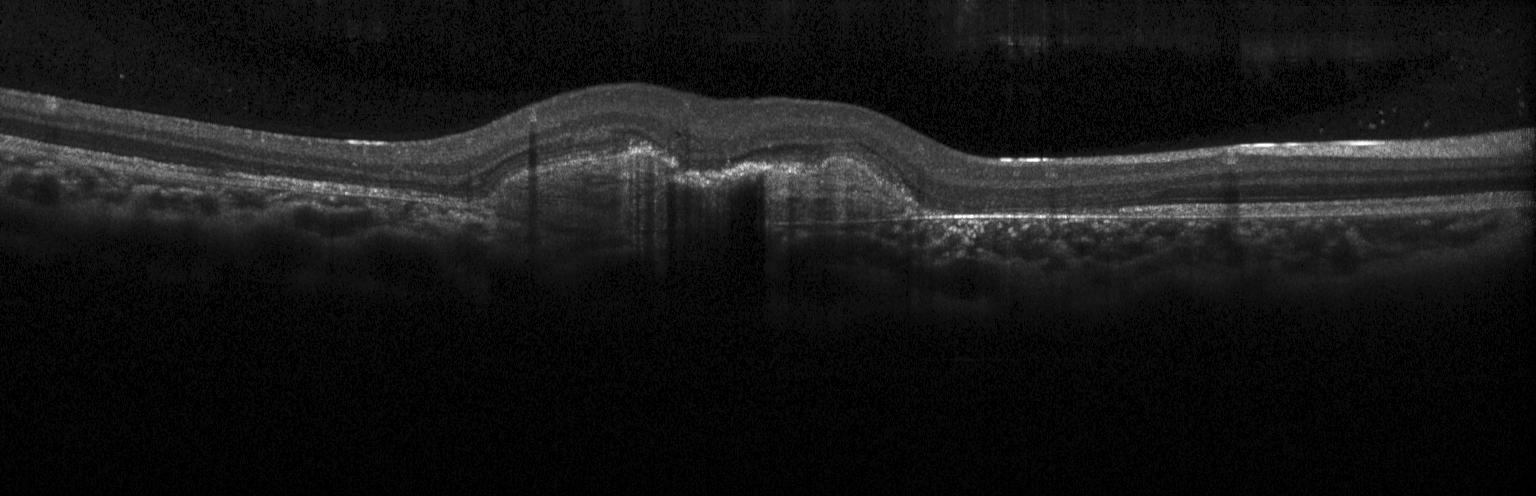

Retinal OCT cross-section.
Dx: choroidal neovascularization.